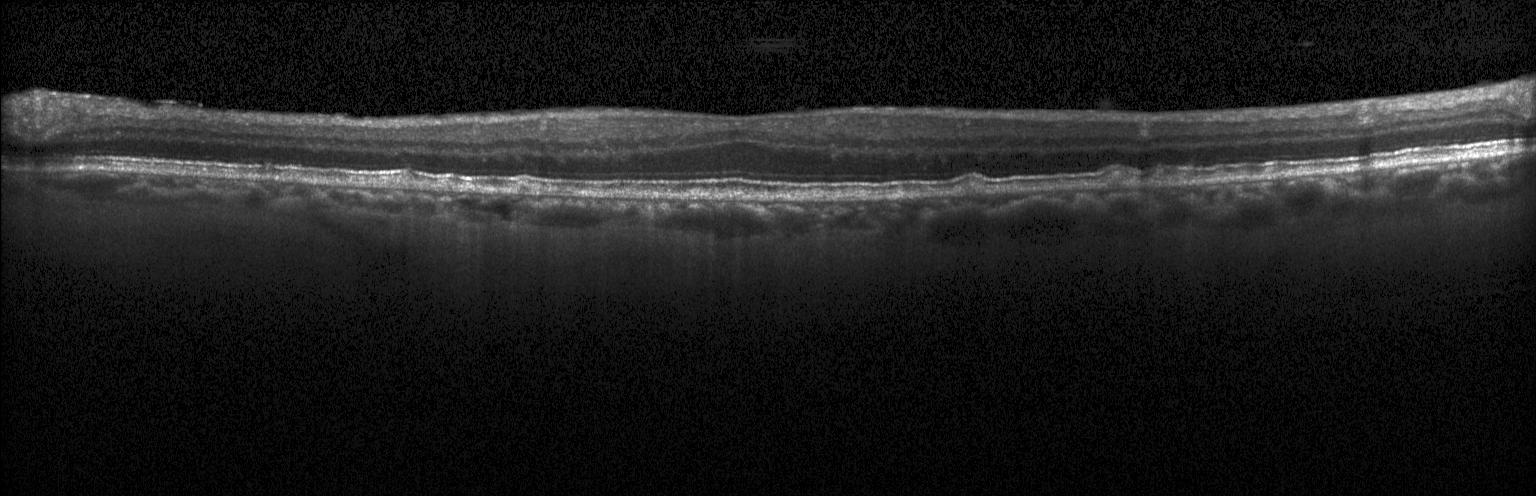

Dx: multiple drusen.